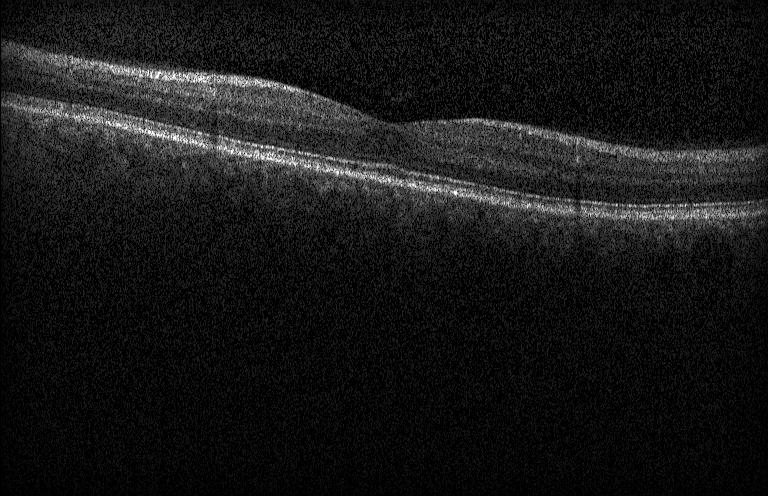
OCT scan showing no choroidal neovascularization, diabetic macular edema, or drusen.